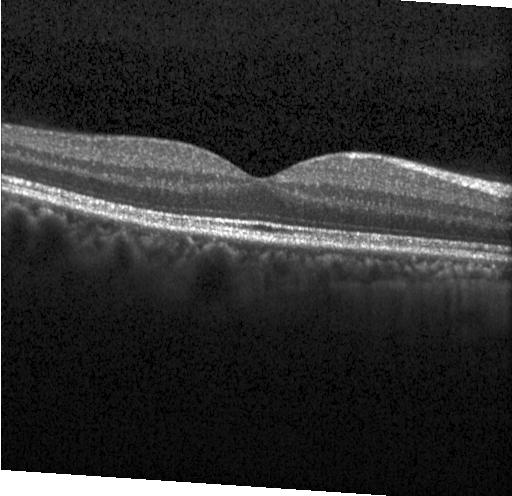

Macular OCT: no choroidal neovascularization, no diabetic macular edema, and no drusen.